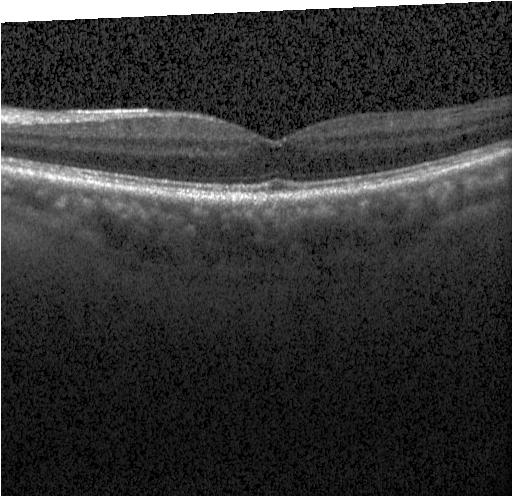
Optical coherence tomography scan — Macular OCT: no choroidal neovascularization, no diabetic macular edema, and no drusen.